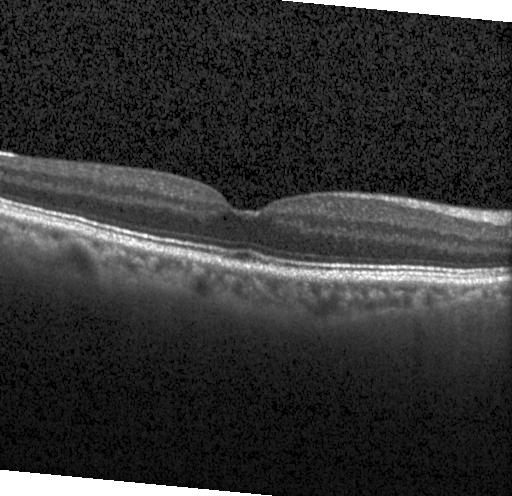
Diagnosis: no choroidal neovascularization, diabetic macular edema, or drusen.